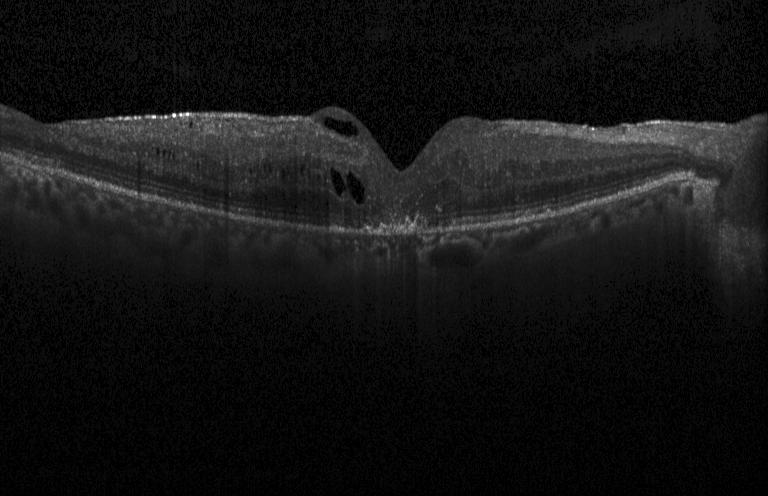

Spectral-domain OCT. Optical coherence tomography scan. Centered on the fovea. Instrument: Heidelberg Spectralis.
Assessment: DME.